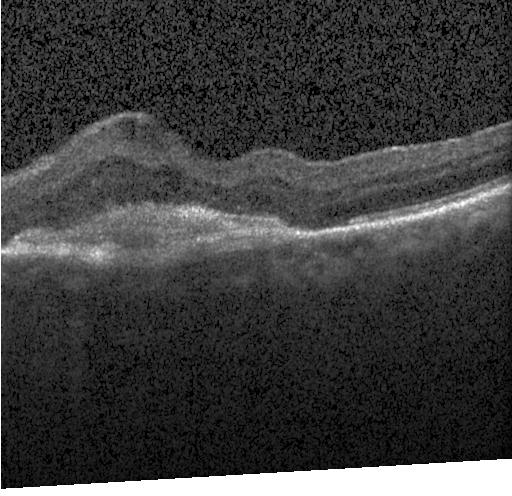 Impression: choroidal neovascularization.